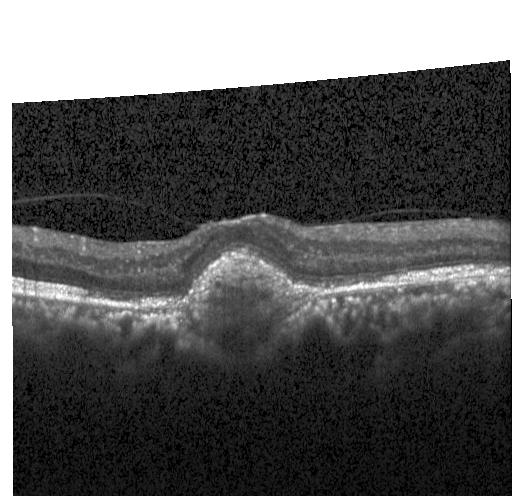 Impression: choroidal neovascularization.